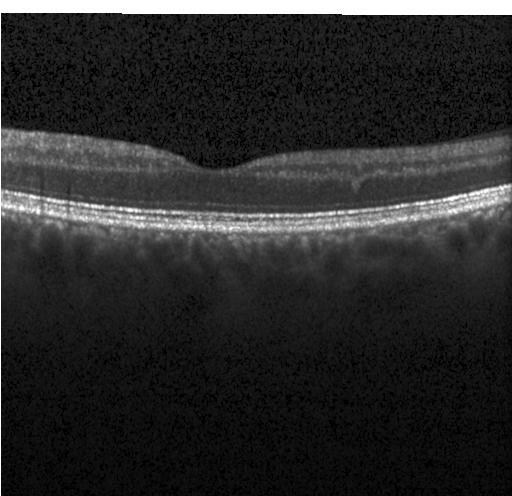
OCT line scan.
No CNV, no DME, and no drusen.